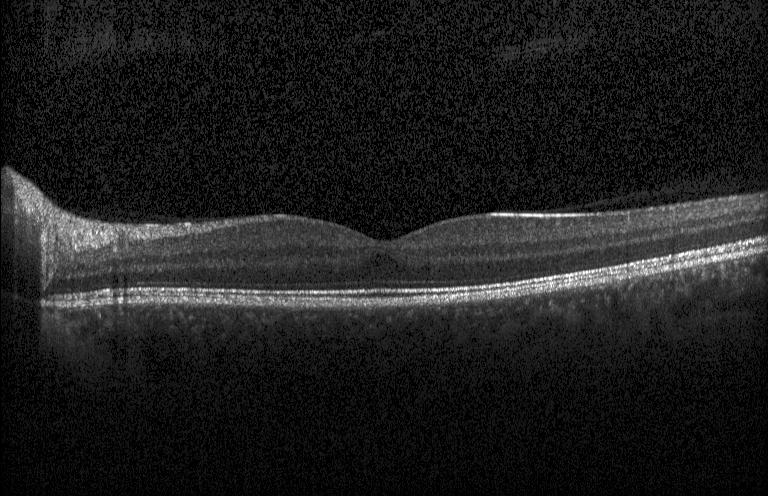
OCT scan showing no choroidal neovascularization, no diabetic macular edema, and no drusen.